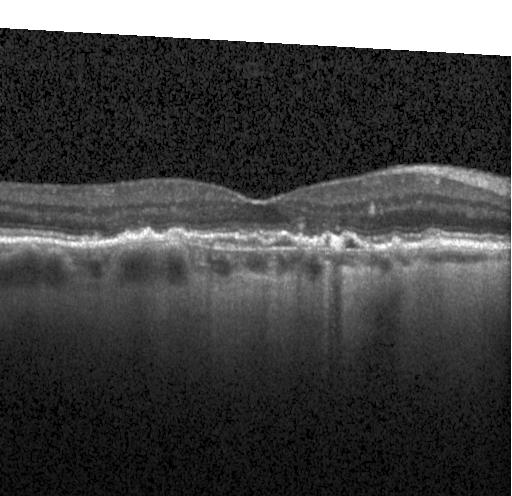

Through the macula; optical coherence tomography B-scan; instrument: Heidelberg Spectralis — Impression: a choroidal neovascular membrane.